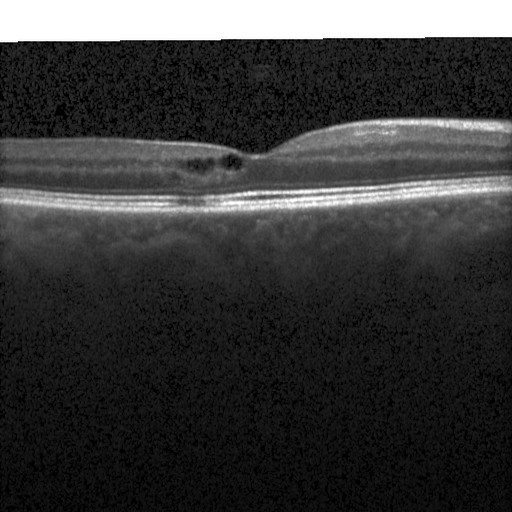
OCT scan showing diabetic macular edema (DME).